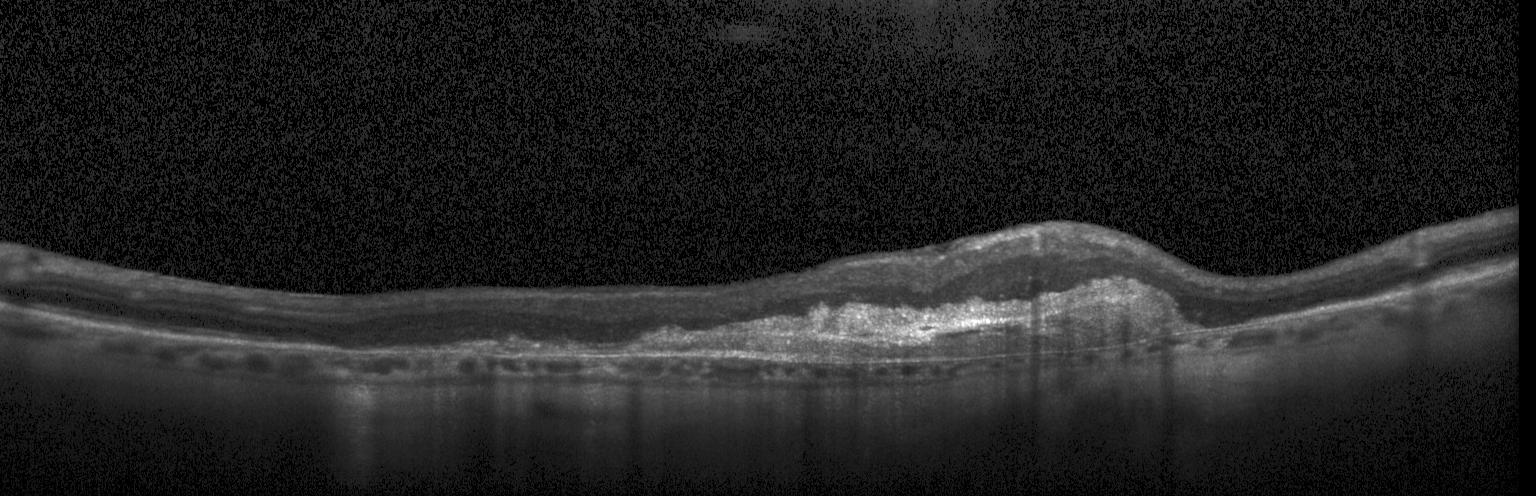

Spectral-domain optical coherence tomography. Heidelberg Spectralis OCT system. OCT line scan
Impression: CNV.